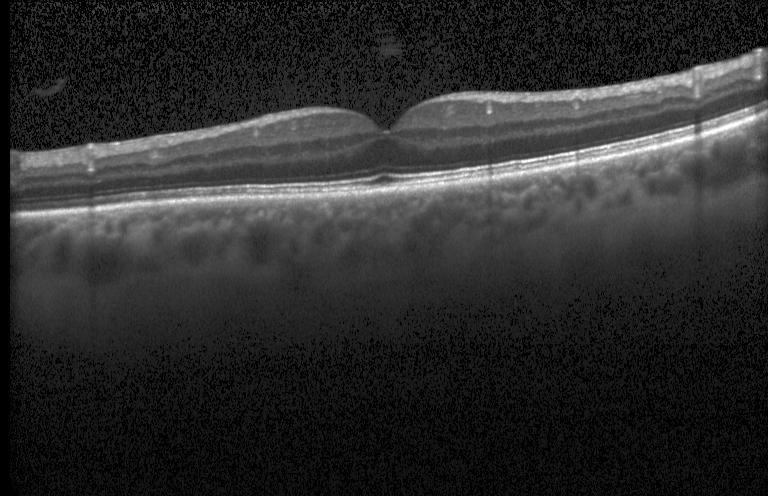 Finding: no evidence of choroidal neovascularization, diabetic macular edema, or drusen.